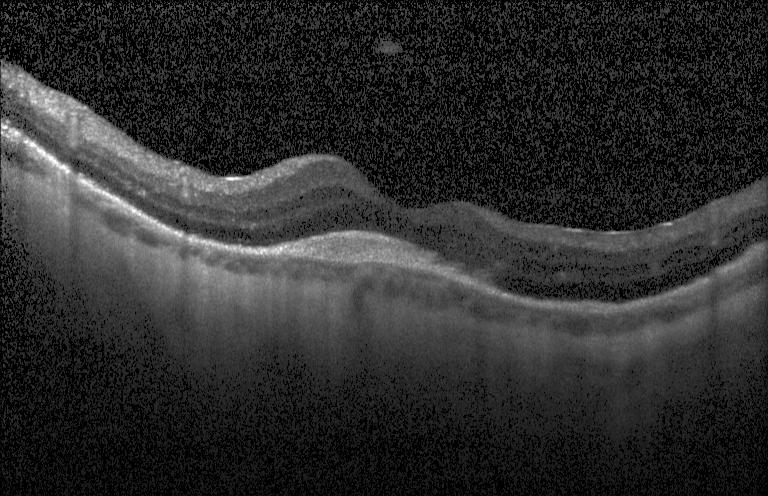
Horizontal scan through the fovea, OCT line scan, spectral-domain optical coherence tomography.
CNV.